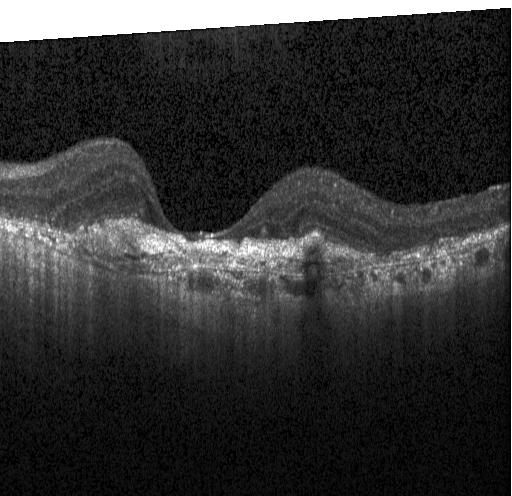 Impression: choroidal neovascularization.